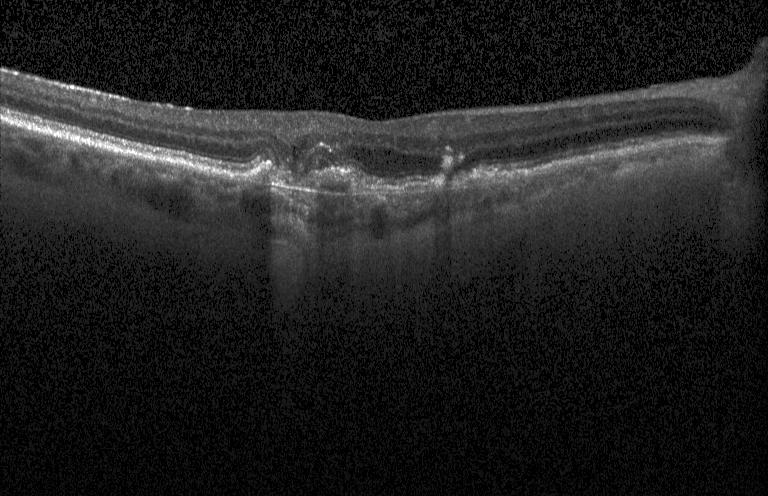
Fovea-centered · OCT B-scan.
Diagnosis: choroidal neovascularization (CNV).